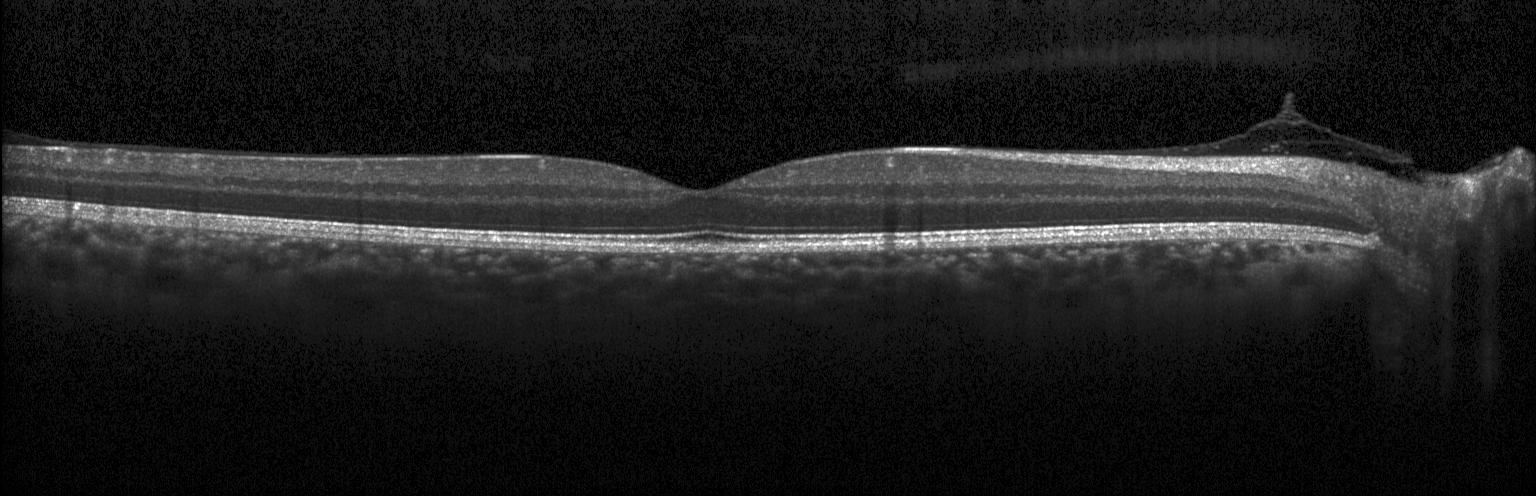 Horizontal scan through the fovea, spectral-domain optical coherence tomography, OCT B-scan, Heidelberg Spectralis.
Finding: no evidence of choroidal neovascularization, diabetic macular edema, or drusen.